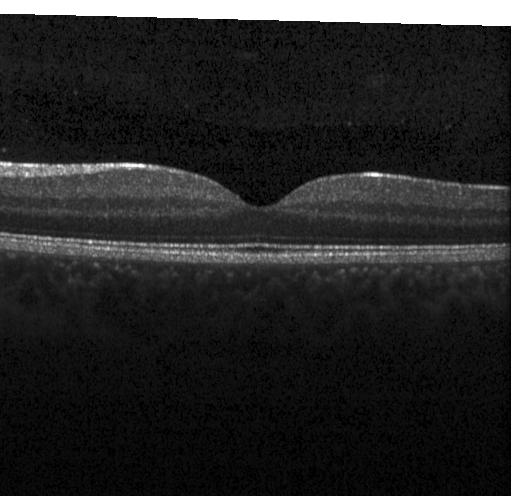 The scan shows neither choroidal neovascularization, diabetic macular edema, nor drusen.